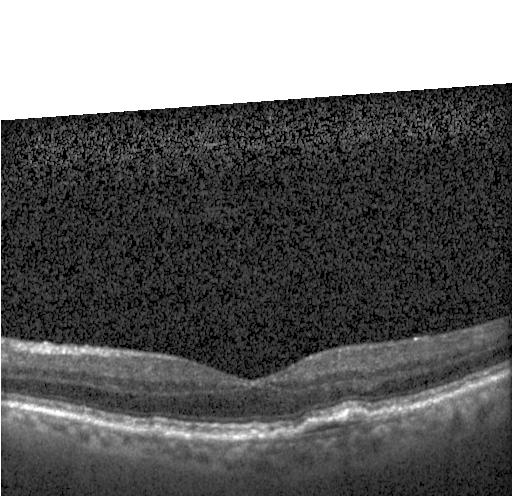
Spectral-domain OCT; macular scan; optical coherence tomography B-scan
Diagnosis: a choroidal neovascular membrane.